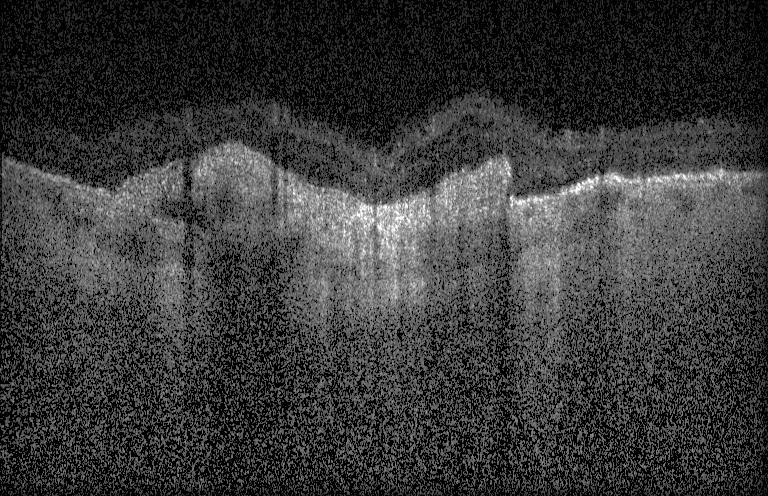
OCT finding: a choroidal neovascular membrane.